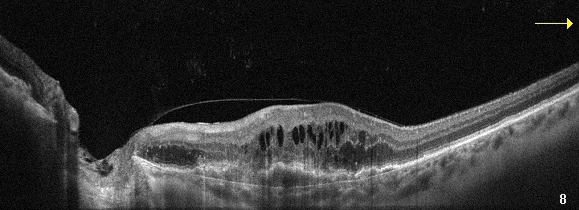 Impression: AMD.